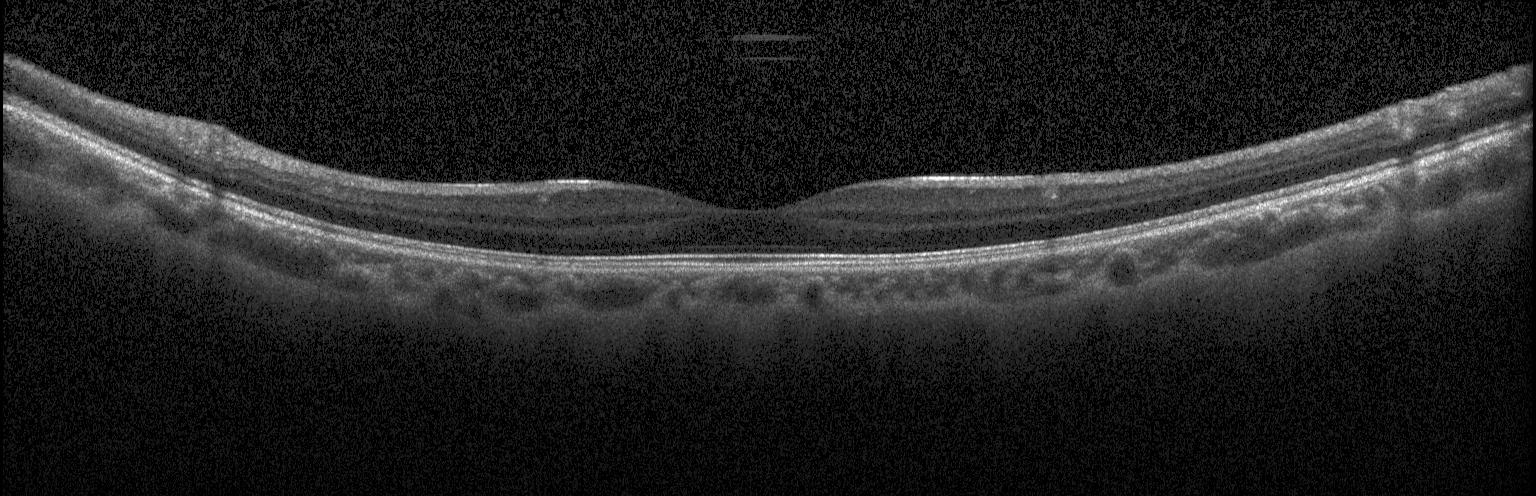
SD-OCT; horizontal scan through the fovea; Heidelberg Spectralis OCT system; OCT B-scan — Assessment: no CNV, DME, or drusen.